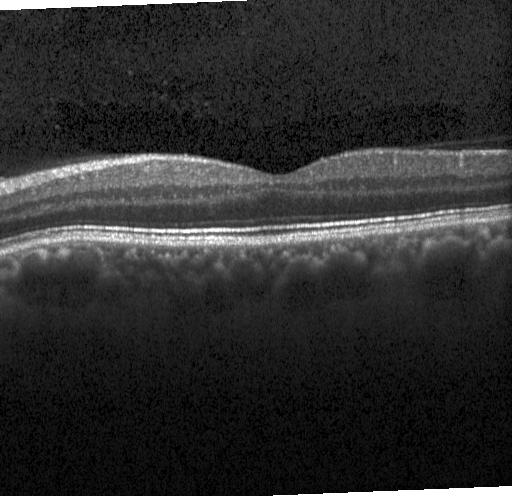 Assessment: no evidence of choroidal neovascularization, diabetic macular edema, or drusen.